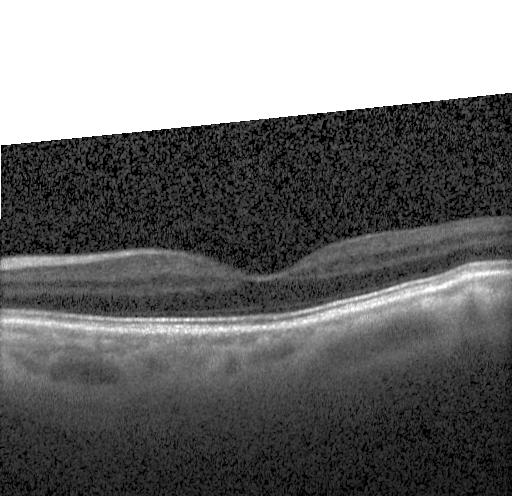

OCT line scan. Diagnosis: no choroidal neovascularization, diabetic macular edema, or drusen.